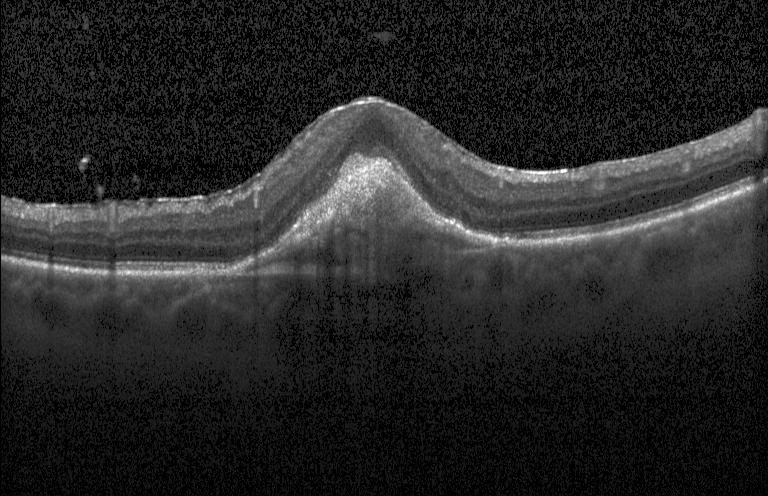

Macular scan, instrument: Heidelberg Spectralis, retinal OCT cross-section. Macular OCT: choroidal neovascularization.